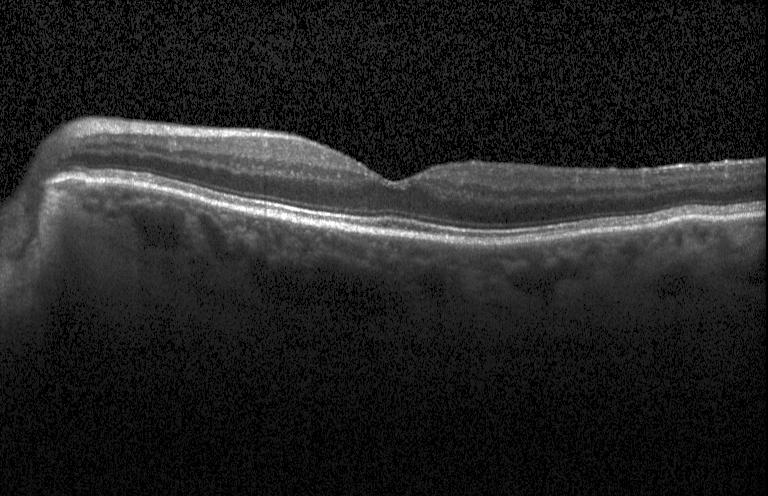
OCT finding: neither CNV, DME, nor drusen.